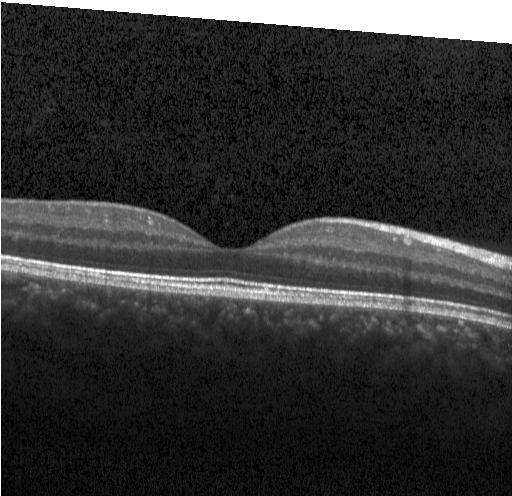

Impression: no CNV, DME, or drusen.